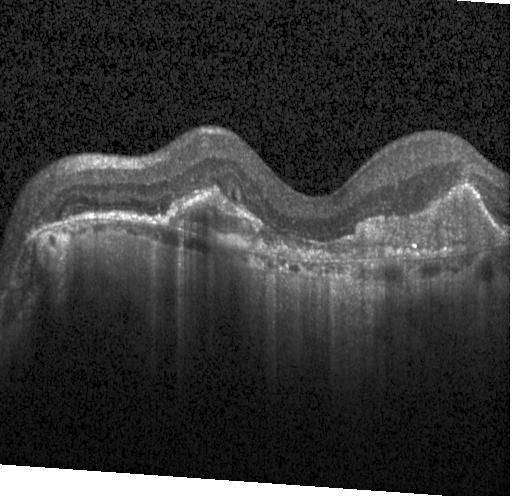
Retinal OCT cross-section · Heidelberg Spectralis OCT system · spectral-domain OCT.
Diagnosis: choroidal neovascularization.